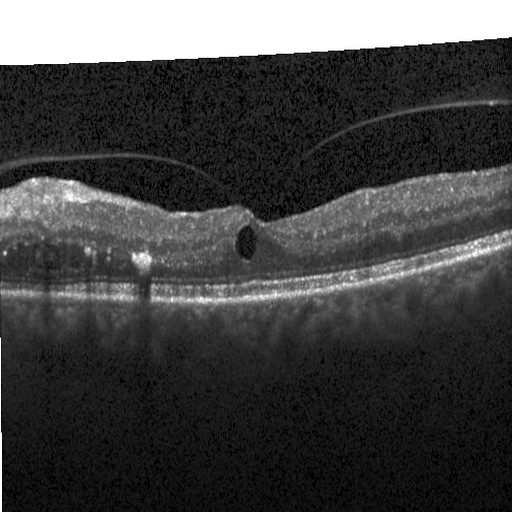
Retinal OCT B-scan
Finding: diabetic macular edema (DME).